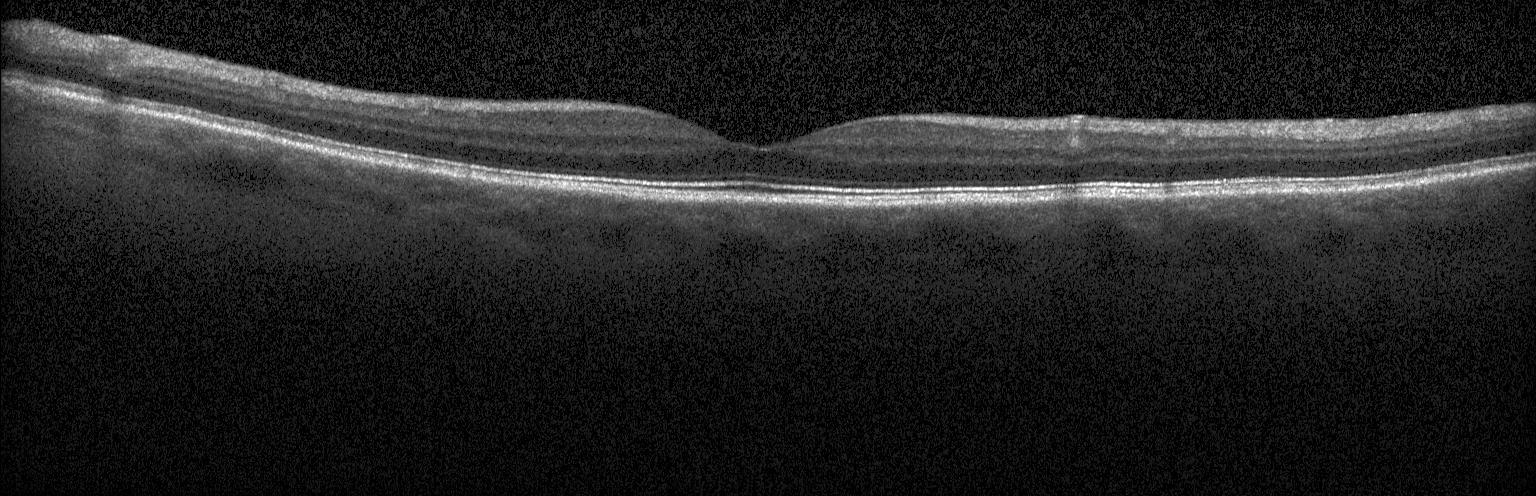 Retinal OCT cross-section — This B-scan demonstrates no evidence of CNV, DME, or drusen.